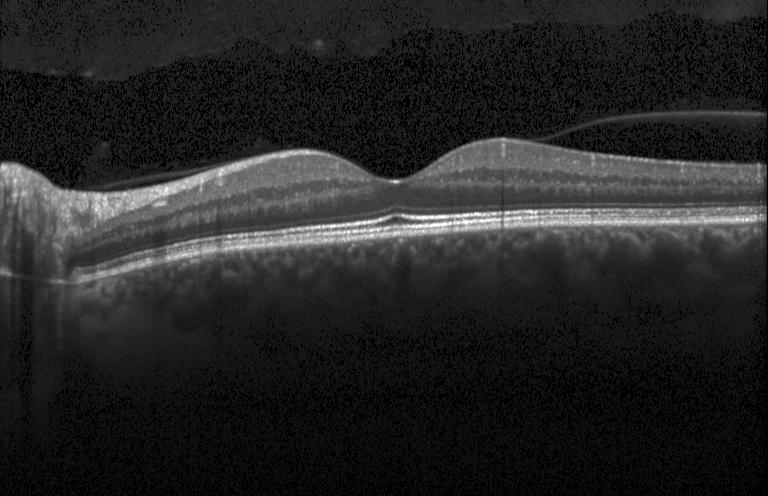

OCT B-scan showing no choroidal neovascularization, no diabetic macular edema, and no drusen.